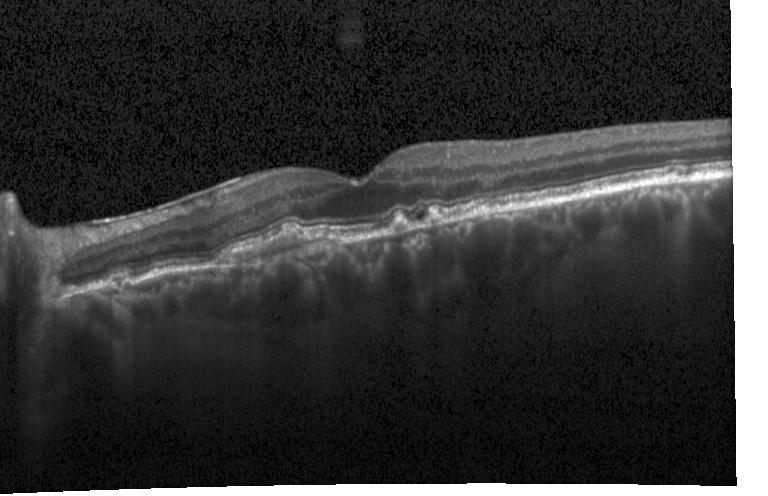

Spectral-domain OCT, retinal OCT cross-section, fovea-centered
Impression: choroidal neovascularization (CNV).